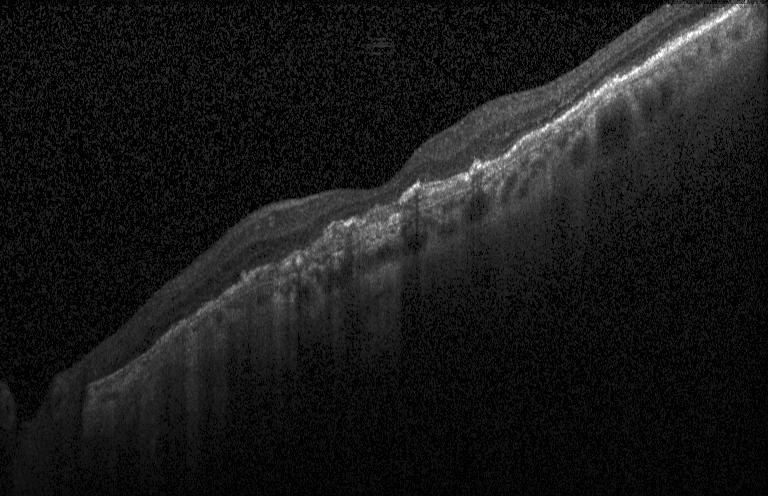 Macular scan; SD-OCT; instrument: Heidelberg Spectralis; optical coherence tomography B-scan
A choroidal neovascular membrane.